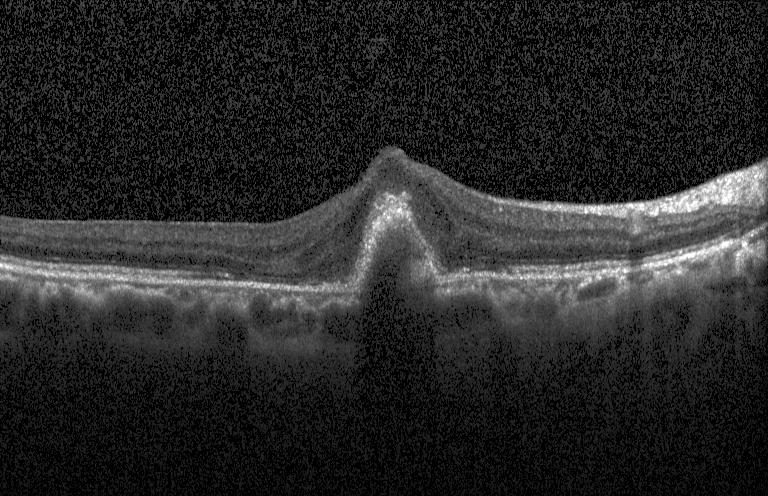 Optical coherence tomography B-scan.
The scan shows CNV.